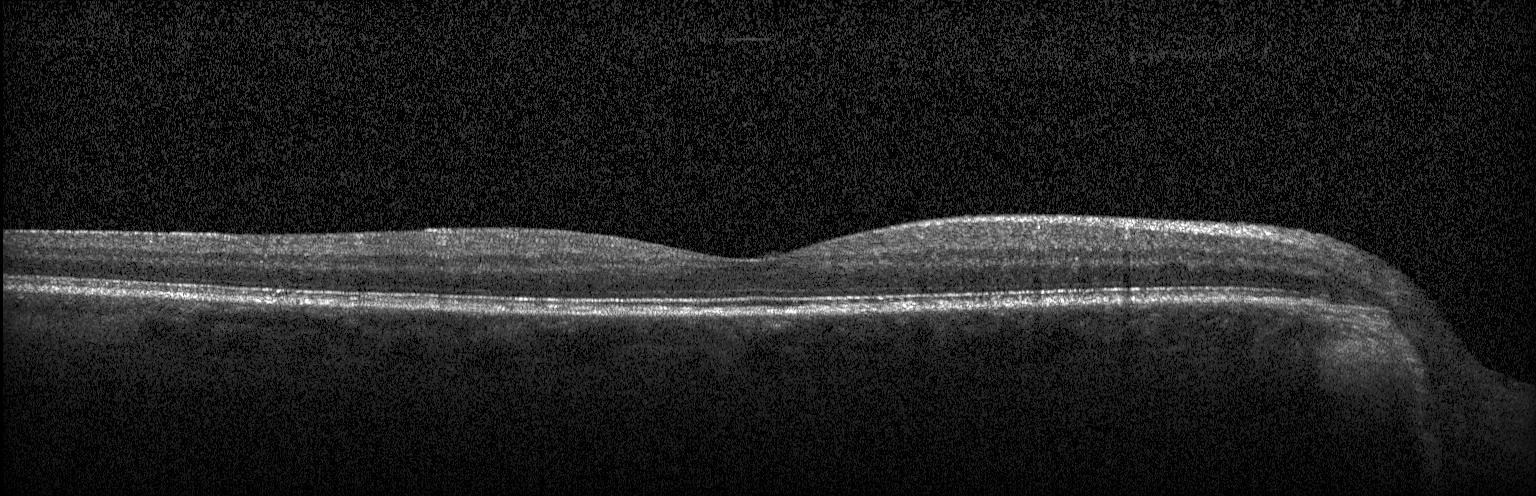
OCT B-scan. Impression: no choroidal neovascularization, no diabetic macular edema, and no drusen.